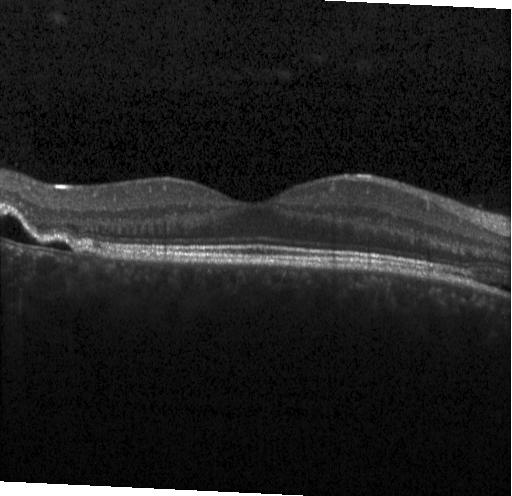
Heidelberg Spectralis OCT system, retinal OCT cross-section, fovea-centered
The scan shows a choroidal neovascular membrane.